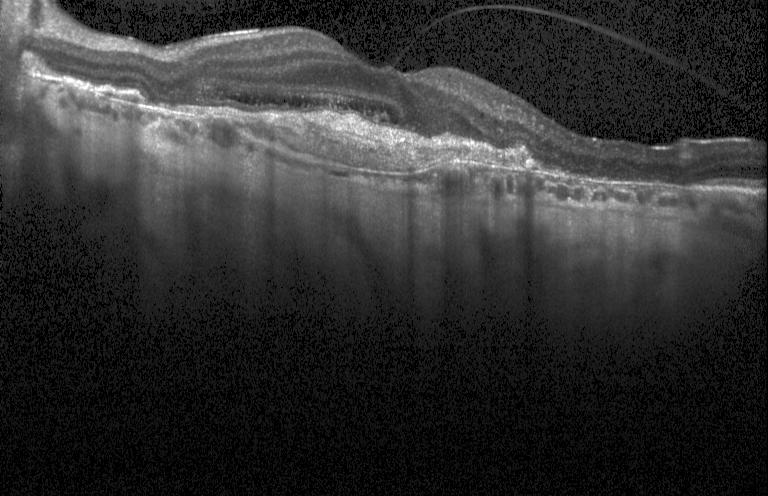
Retinal OCT cross-section, centered on the fovea, instrument: Heidelberg Spectralis
Impression: choroidal neovascularization (CNV).